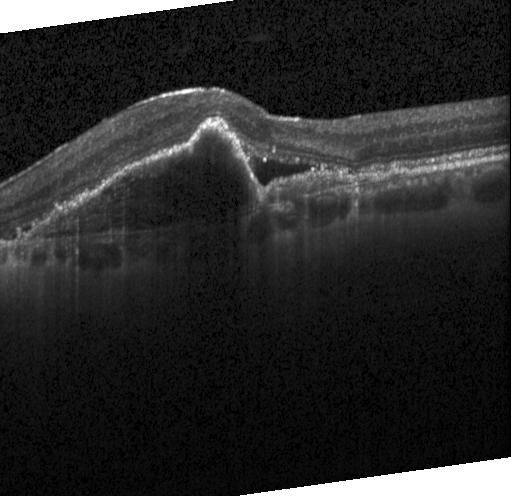 Retinal OCT cross-section — OCT finding: choroidal neovascularization.